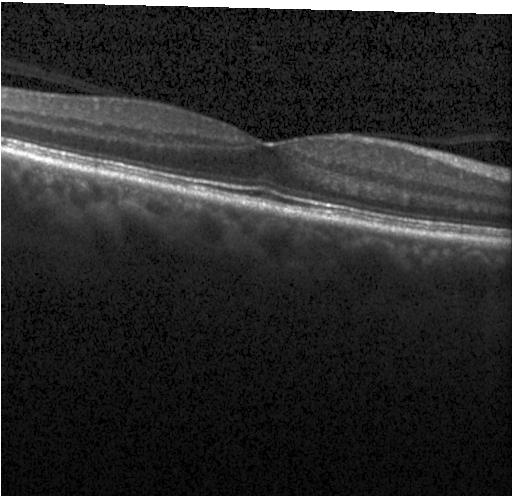 OCT B-scan · through the macula. Diagnosis: no choroidal neovascularization, no diabetic macular edema, and no drusen.